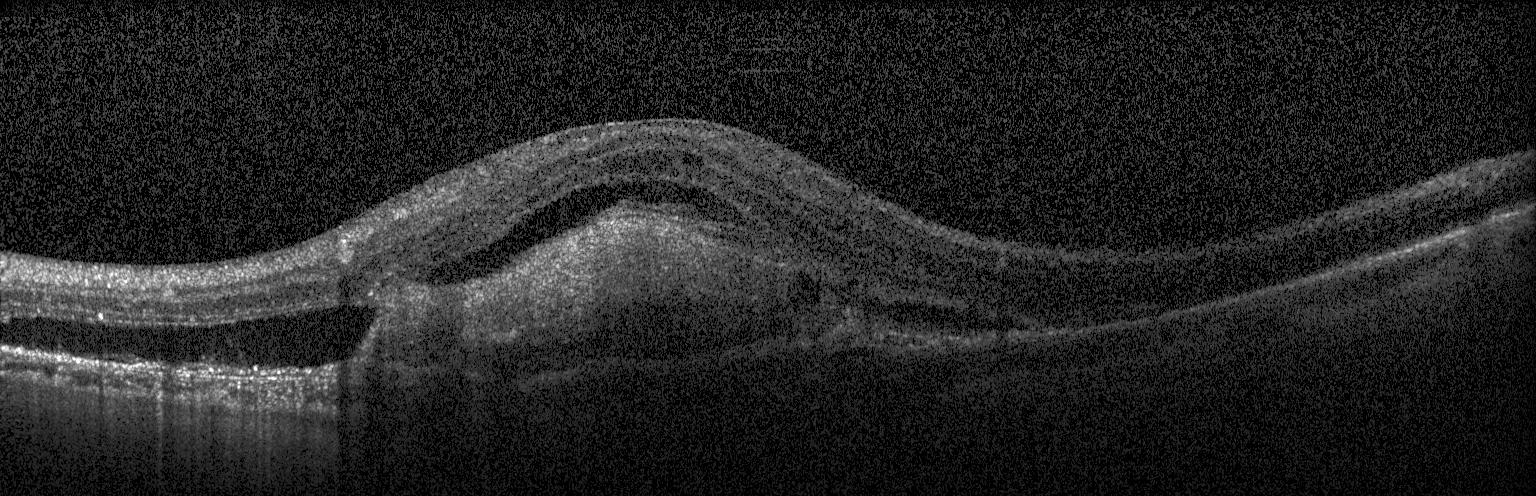

Spectral-domain OCT B-scan: choroidal neovascularization.